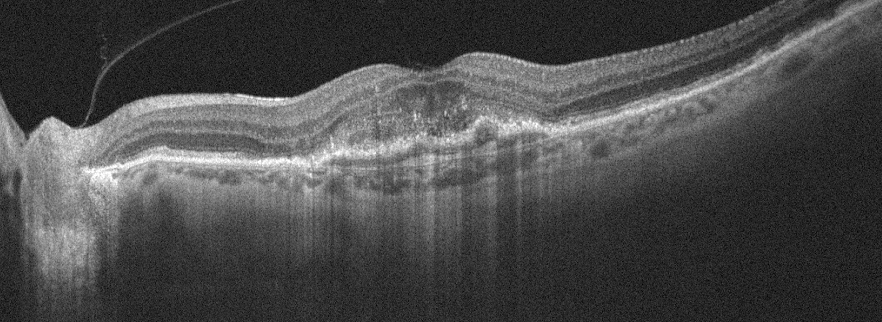
Retinal OCT B-scan, macular scan, Optovue Avanti RTVue XR. Macular OCT: age-related macular degeneration (AMD).